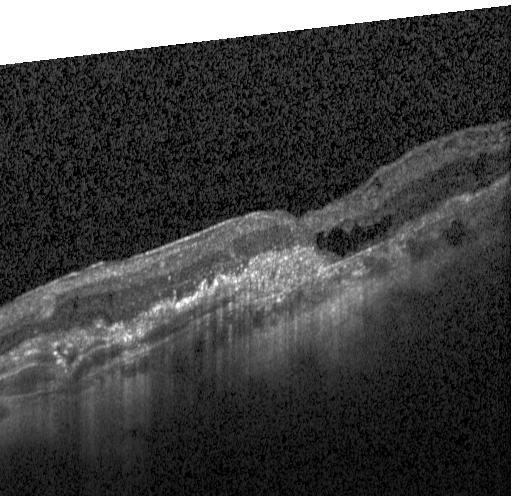
Impression: a choroidal neovascular membrane.